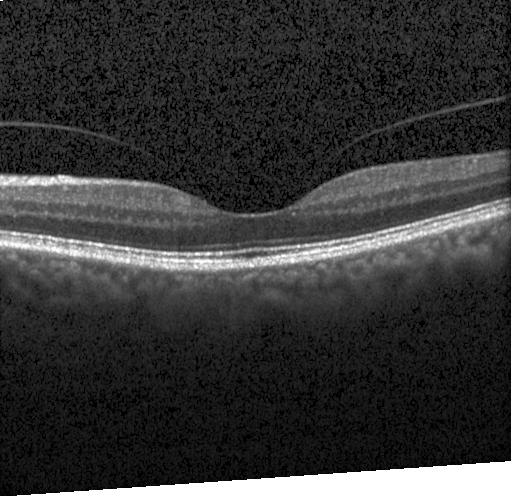

Retinal OCT B-scan — Finding: no evidence of CNV, DME, or drusen.